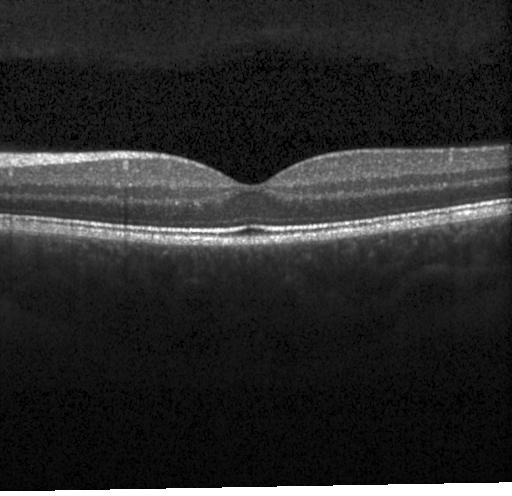

Retinal OCT cross-section
This B-scan demonstrates neither CNV, DME, nor drusen.